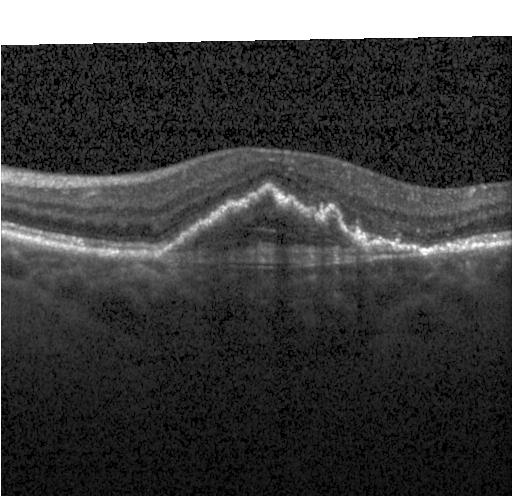
Retinal OCT cross-section. Instrument: Heidelberg Spectralis. Horizontal scan through the fovea. Finding: choroidal neovascularization (CNV).